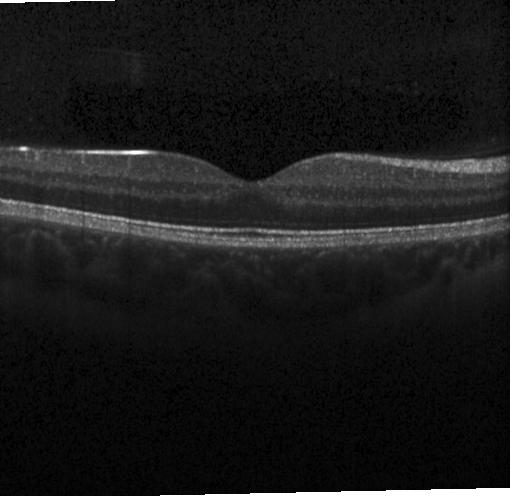
Diagnosis: neither choroidal neovascularization, diabetic macular edema, nor drusen.